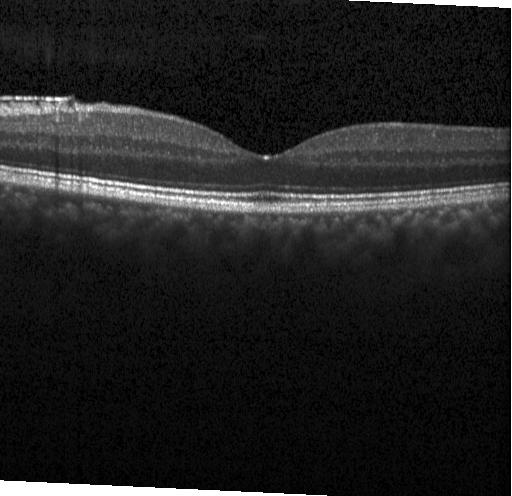 Assessment: no choroidal neovascularization, no diabetic macular edema, and no drusen.